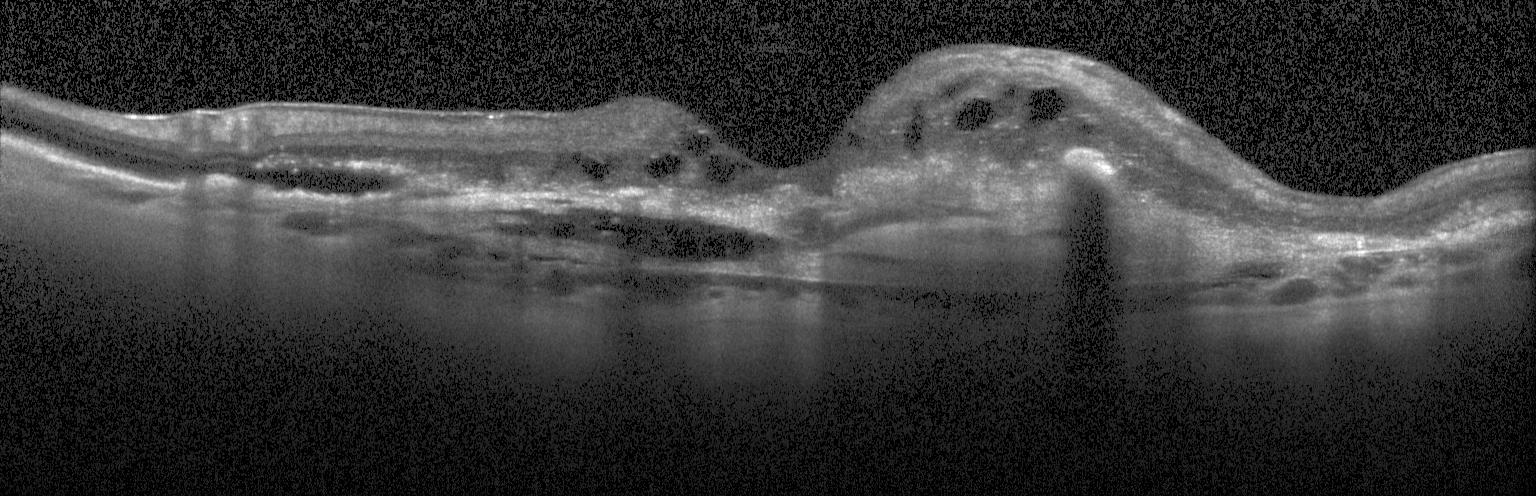 Heidelberg Spectralis; optical coherence tomography scan; SD-OCT. Impression: choroidal neovascularization (CNV).